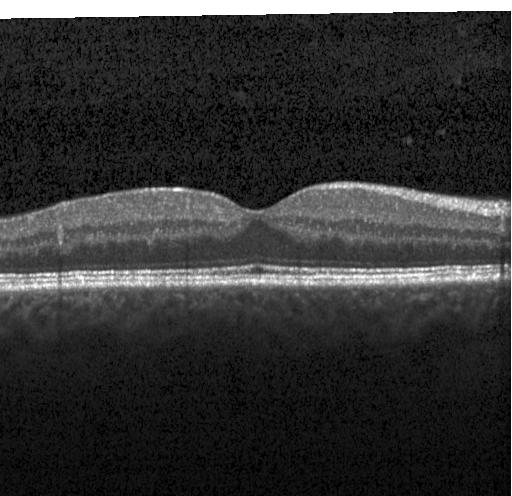
OCT line scan · spectral-domain optical coherence tomography — Impression: no evidence of CNV, DME, or drusen.